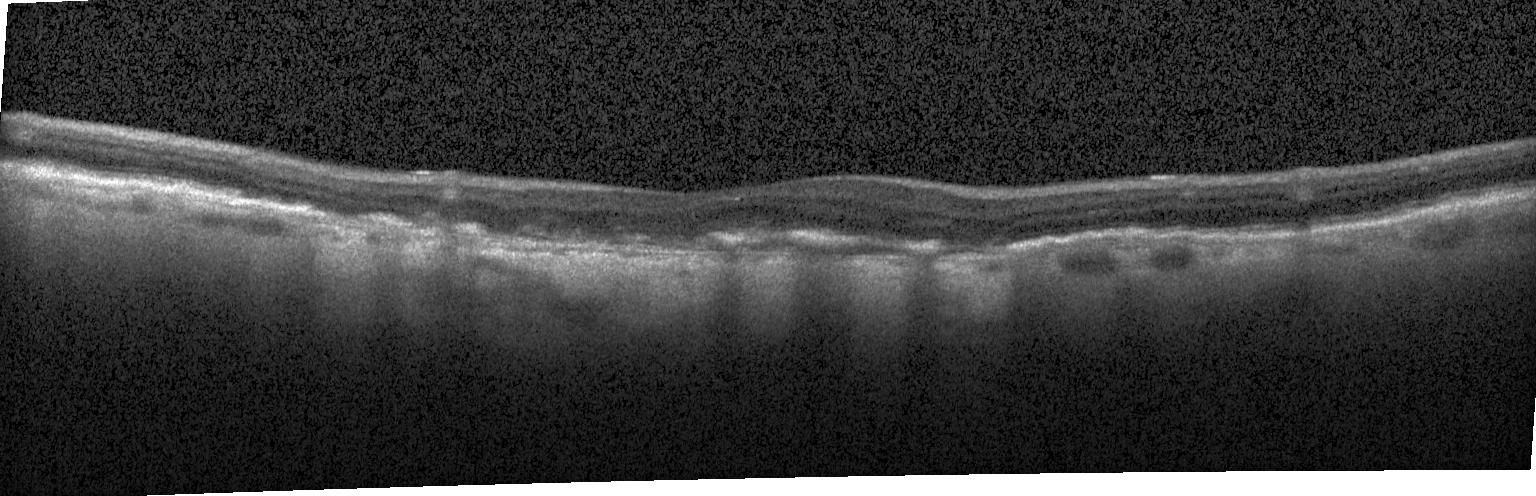

Heidelberg Spectralis OCT system; through the macula; OCT B-scan; spectral-domain optical coherence tomography.
Diagnosis: a choroidal neovascular membrane.